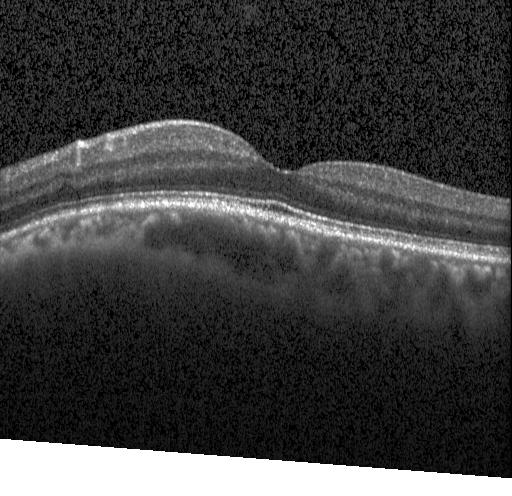

Optical coherence tomography B-scan, through the macula, Heidelberg Spectralis OCT system.
Dx: no choroidal neovascularization, no diabetic macular edema, and no drusen.